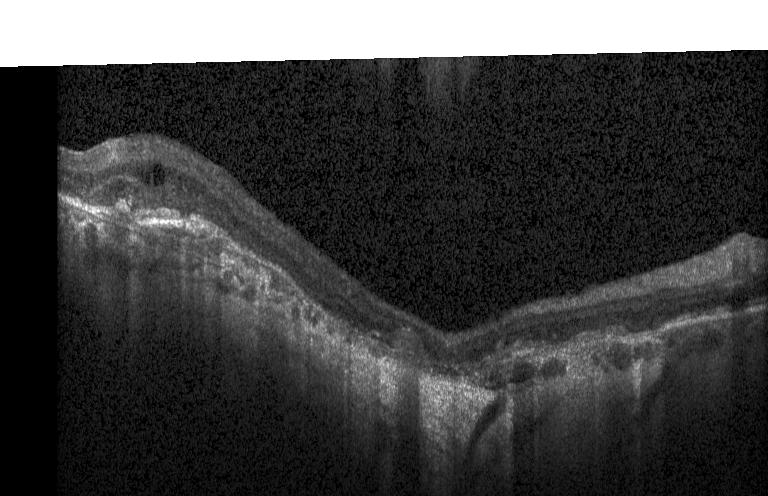

A choroidal neovascular membrane.